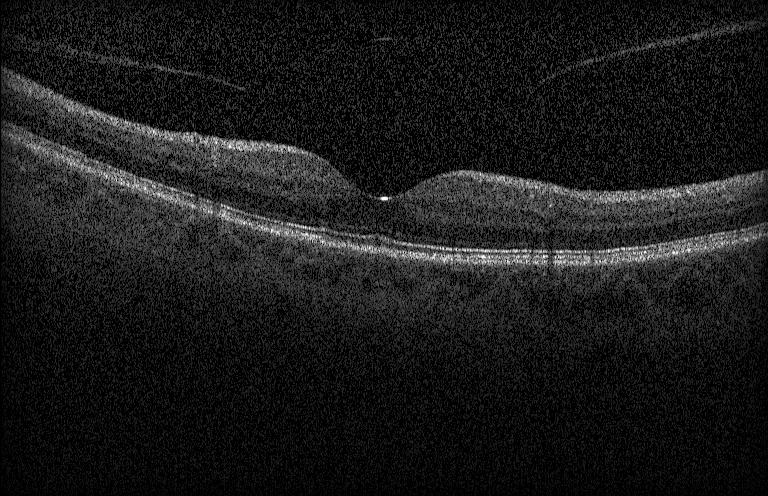 OCT finding: no CNV, DME, or drusen.